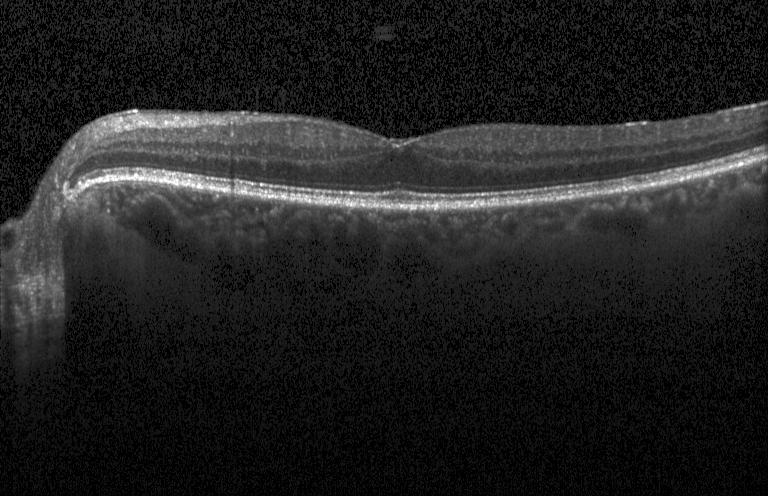 Heidelberg Spectralis. Through the macula. Spectral-domain OCT. Retinal OCT cross-section — The scan shows no evidence of CNV, DME, or drusen.